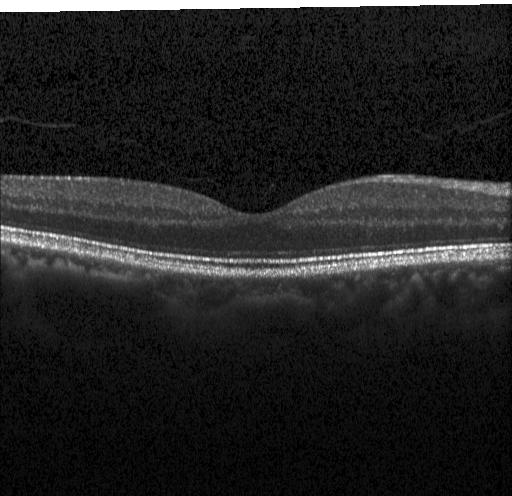

Macular scan · spectral-domain optical coherence tomography · OCT B-scan
This B-scan demonstrates no evidence of choroidal neovascularization, diabetic macular edema, or drusen.